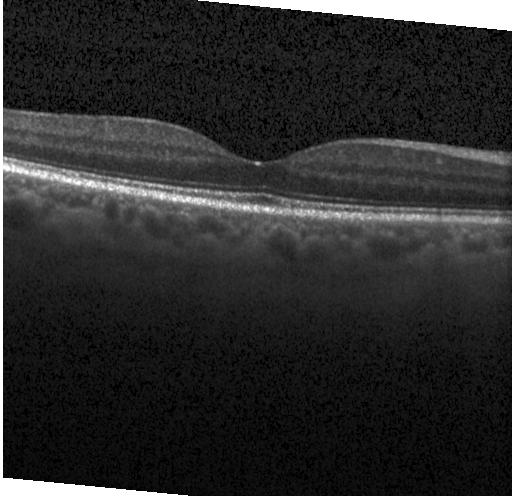
OCT B-scan. This B-scan demonstrates neither choroidal neovascularization, diabetic macular edema, nor drusen.